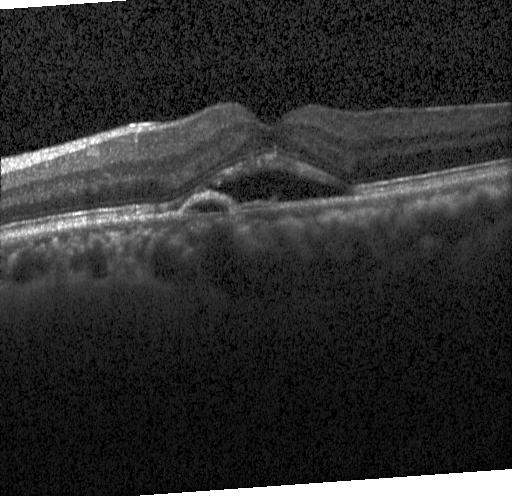
OCT finding: choroidal neovascularization (CNV).